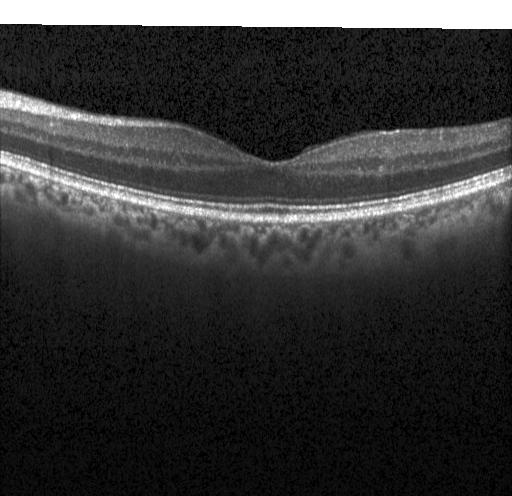

Optical coherence tomography B-scan — Finding: neither CNV, DME, nor drusen.